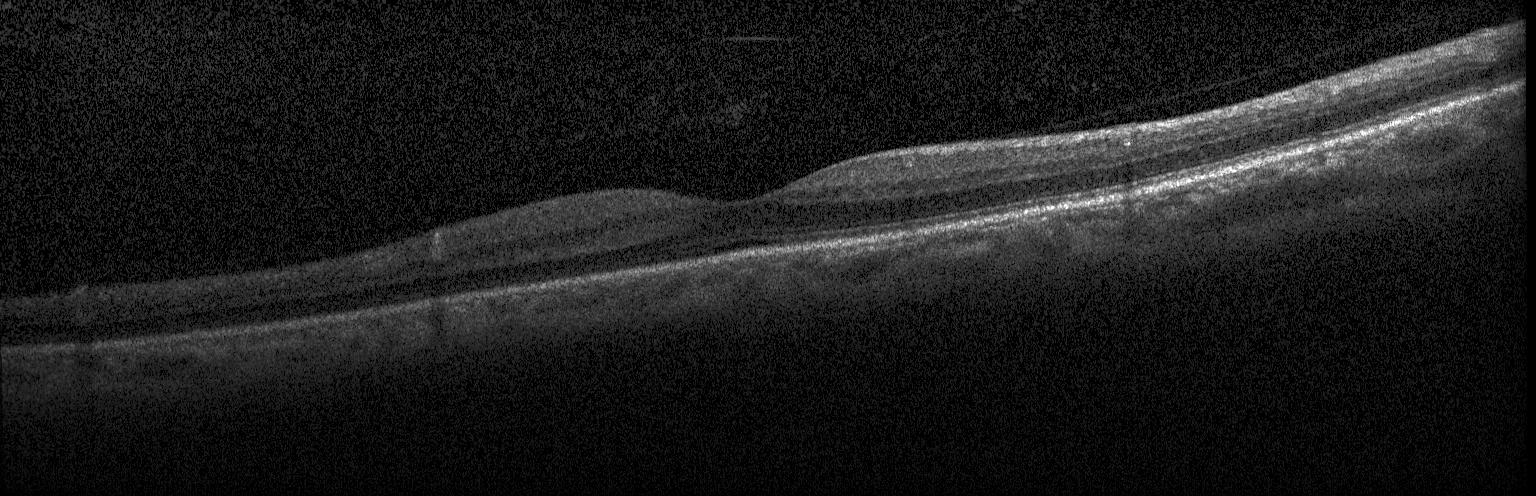
Horizontal scan through the fovea, Heidelberg Spectralis OCT system, retinal OCT cross-section, spectral-domain OCT.
Impression: no CNV, no DME, and no drusen.